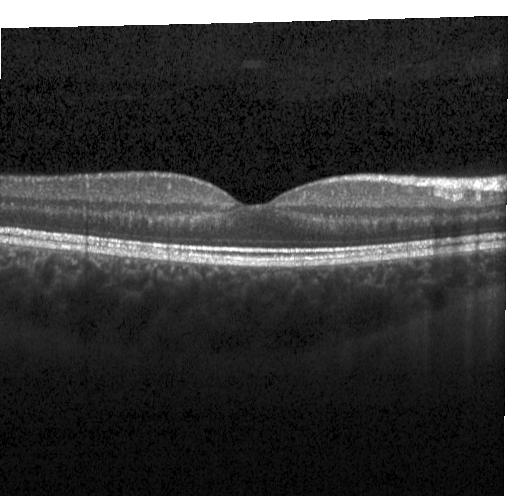 OCT B-scan
Impression: no evidence of CNV, DME, or drusen.